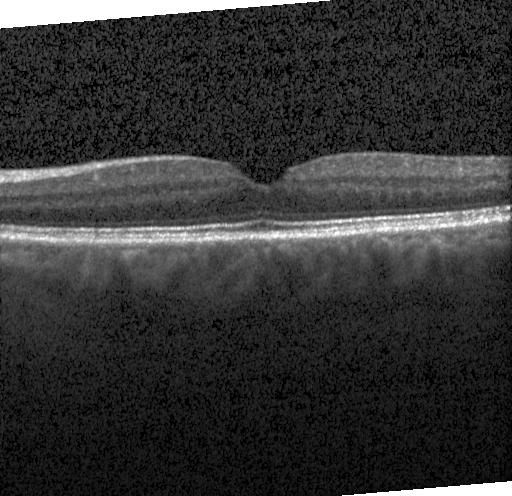 The scan shows no CNV, DME, or drusen.